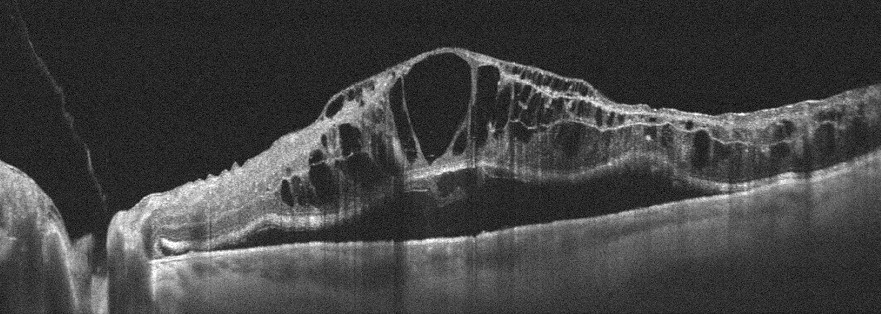 Optovue Avanti RTVue XR; fovea-centered; optical coherence tomography scan — This B-scan demonstrates RVO.